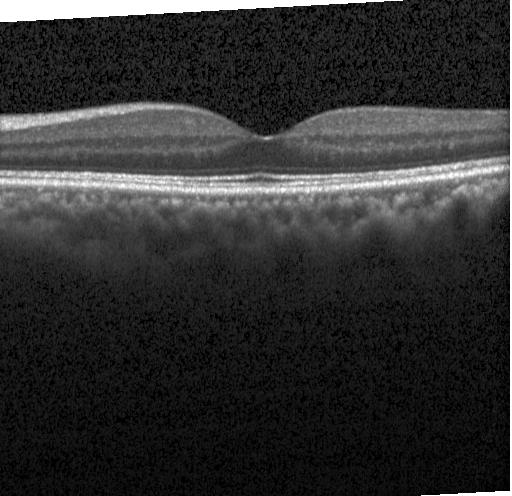

Macular OCT: no evidence of CNV, DME, or drusen.